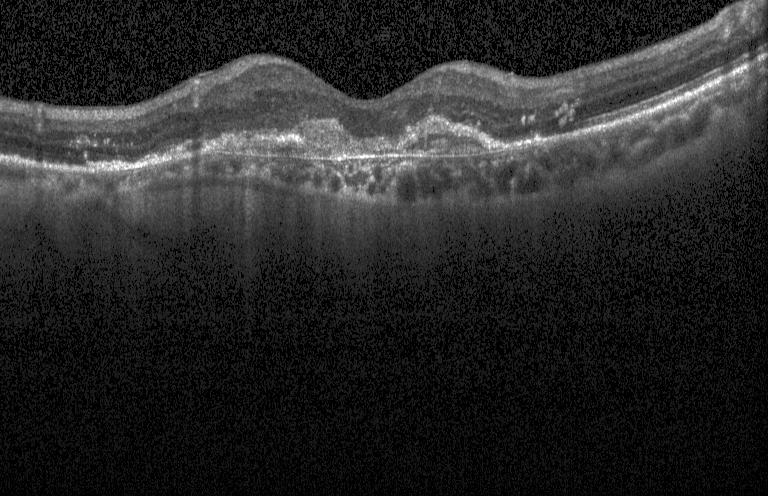

Horizontal scan through the fovea, retinal OCT cross-section. Choroidal neovascularization.